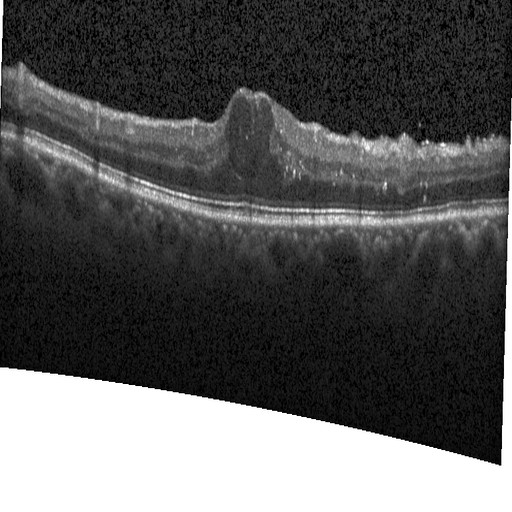 Centered on the fovea. Spectral-domain OCT. Retinal OCT B-scan. Assessment: diabetic macular edema (DME).